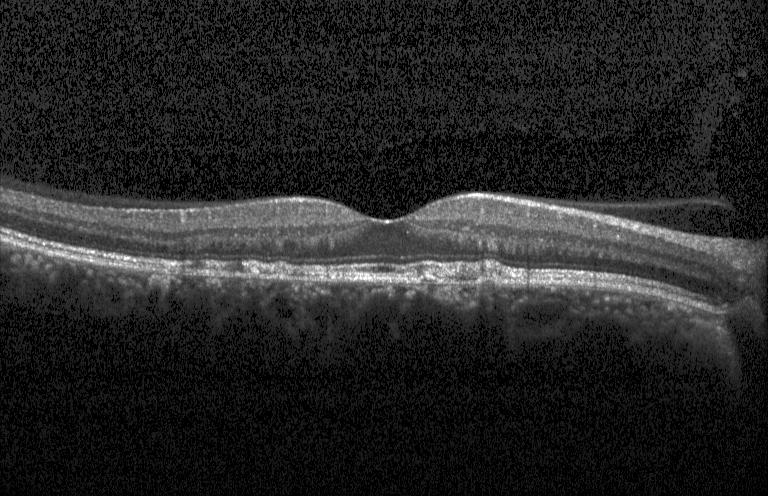
SD-OCT, through the macula, retinal OCT B-scan, acquired on a Heidelberg Spectralis.
The scan shows sub-RPE drusenoid deposits.